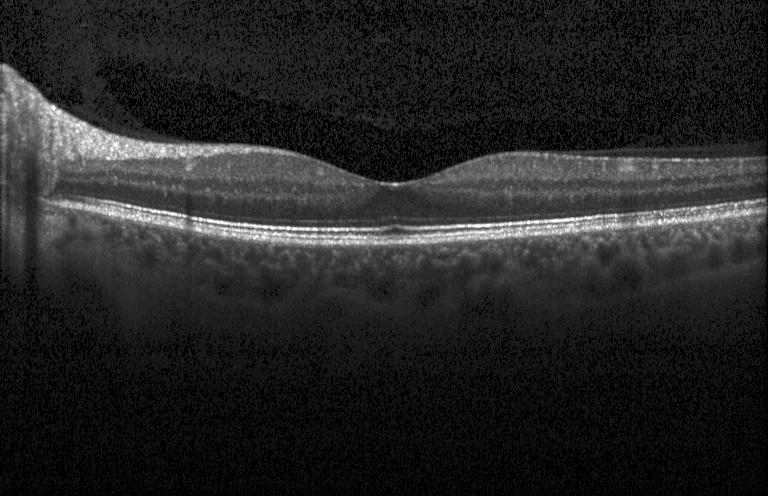

Spectral-domain optical coherence tomography · Heidelberg Spectralis OCT system · OCT B-scan — No CNV, DME, or drusen.